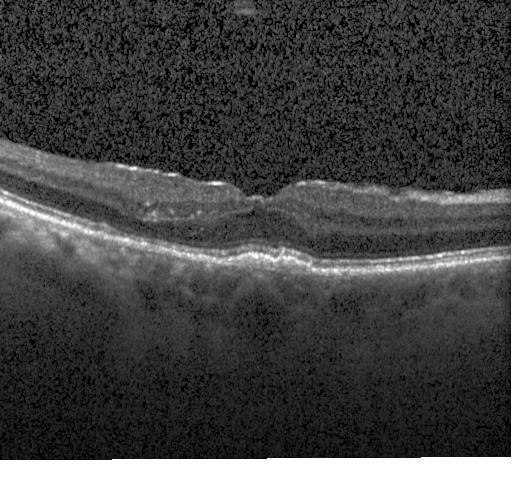

Macular OCT demonstrating a choroidal neovascular membrane.